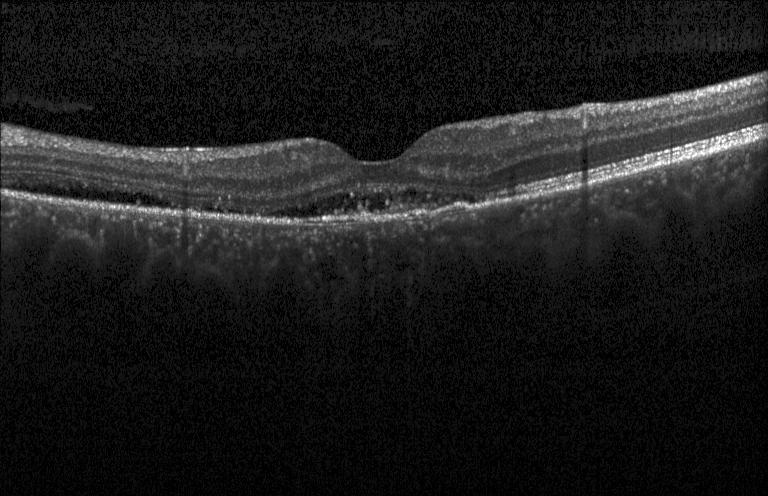

Retinal OCT B-scan
Finding: a choroidal neovascular membrane.